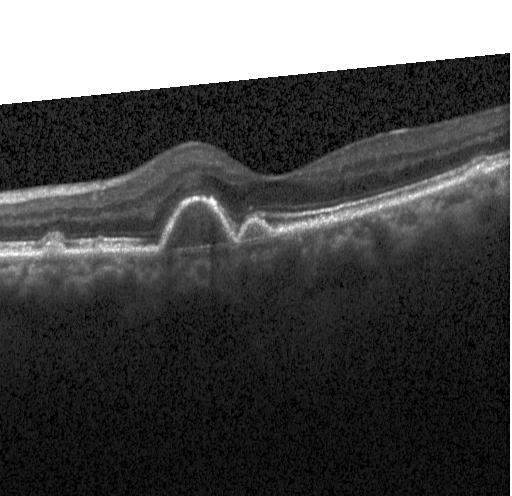
Through the macula. Heidelberg Spectralis OCT system. OCT line scan
The scan shows drusen.